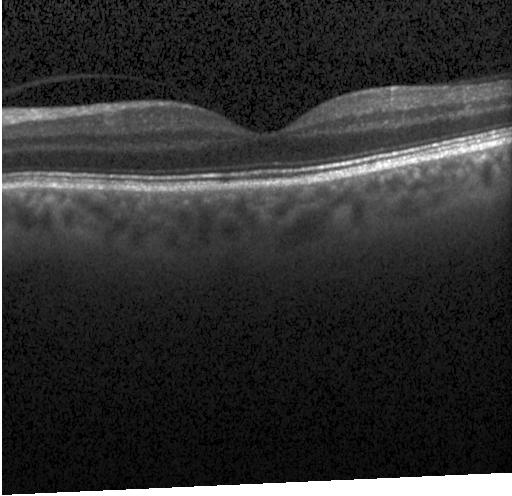
Optical coherence tomography B-scan
The scan shows no CNV, no DME, and no drusen.